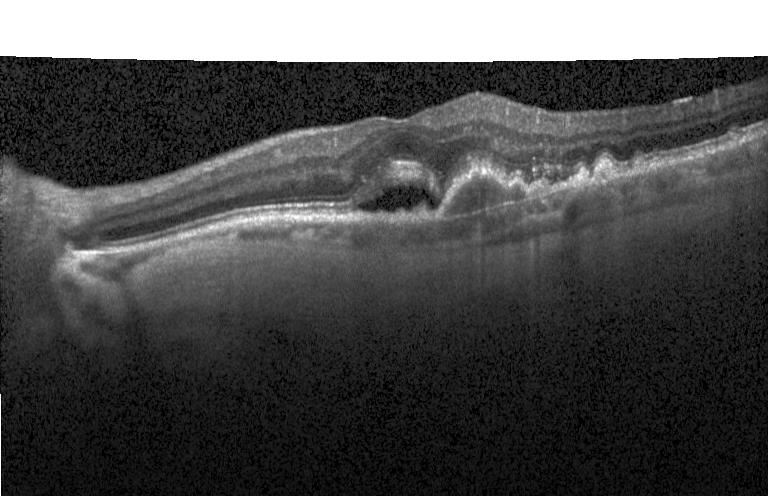

SD-OCT · Heidelberg Spectralis · horizontal scan through the fovea · OCT line scan — Diagnosis: CNV.